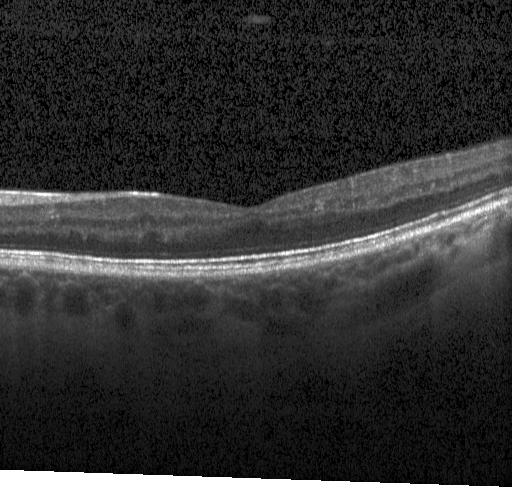

Spectral-domain OCT, macular scan, optical coherence tomography scan, acquired on a Heidelberg Spectralis. The scan shows no choroidal neovascularization, no diabetic macular edema, and no drusen.